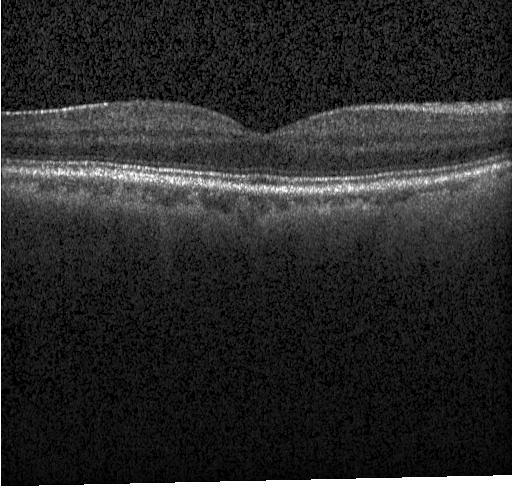
Centered on the fovea, spectral-domain optical coherence tomography, optical coherence tomography B-scan, acquired on a Heidelberg Spectralis.
Finding: no choroidal neovascularization, diabetic macular edema, or drusen.